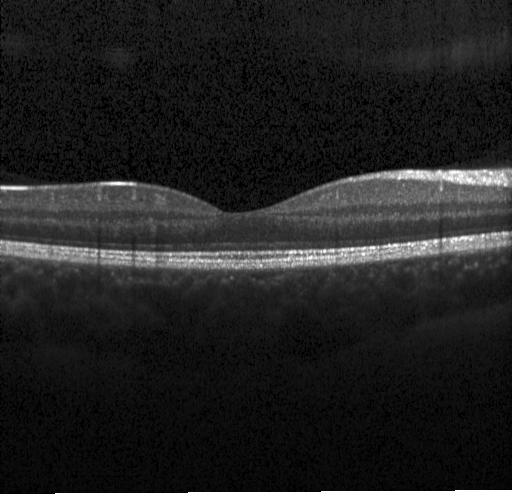
Dx: no CNV, DME, or drusen.